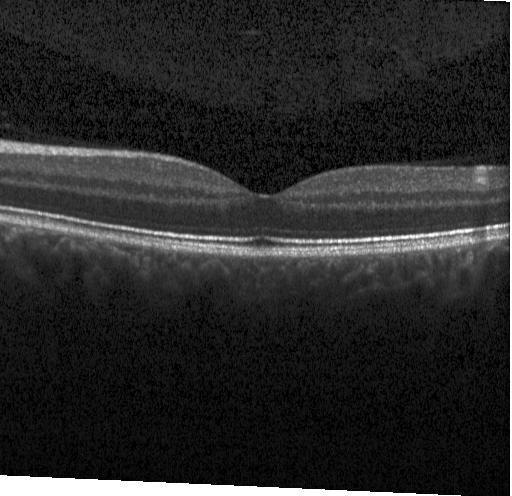 Macular OCT: no choroidal neovascularization, no diabetic macular edema, and no drusen.